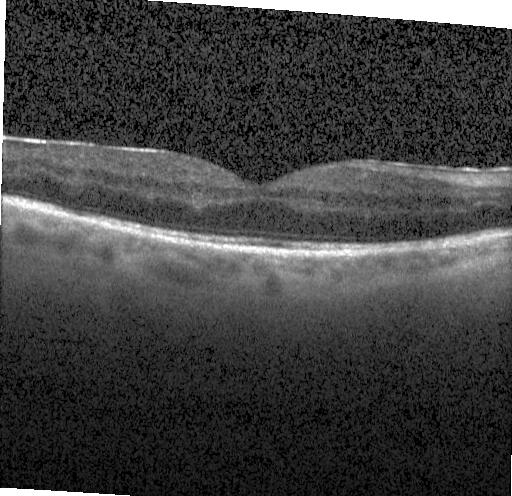 SD-OCT · retinal OCT B-scan. Impression: neither CNV, DME, nor drusen.